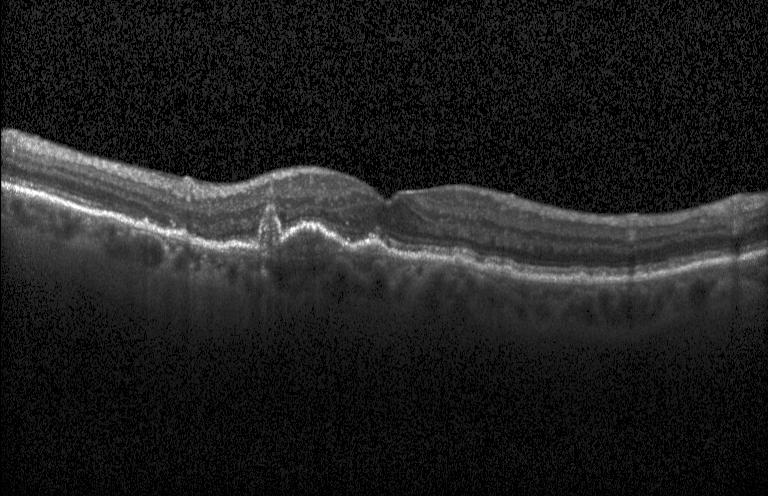

Macular OCT demonstrating choroidal neovascularization.